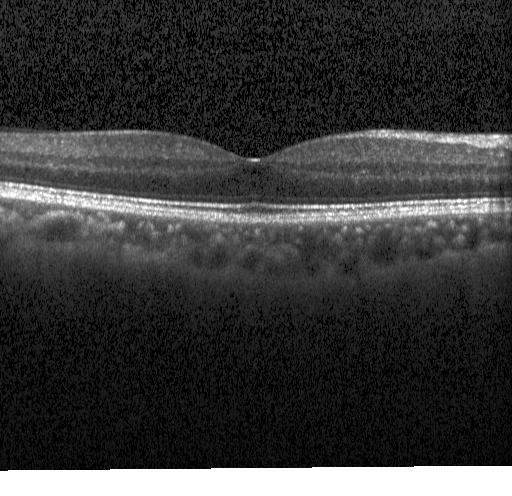 OCT line scan; spectral-domain OCT; fovea-centered; Heidelberg Spectralis
Diagnosis: no choroidal neovascularization, no diabetic macular edema, and no drusen.